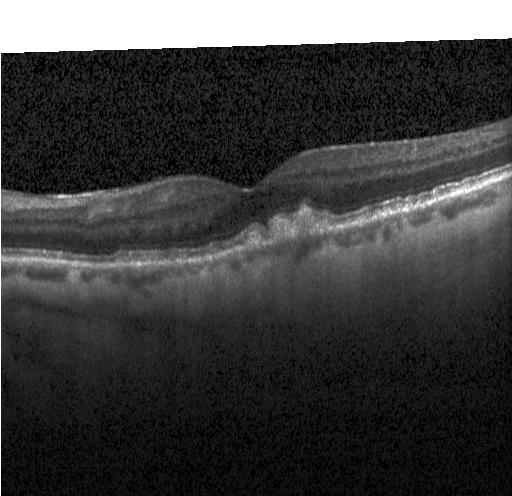
OCT finding: drusen.